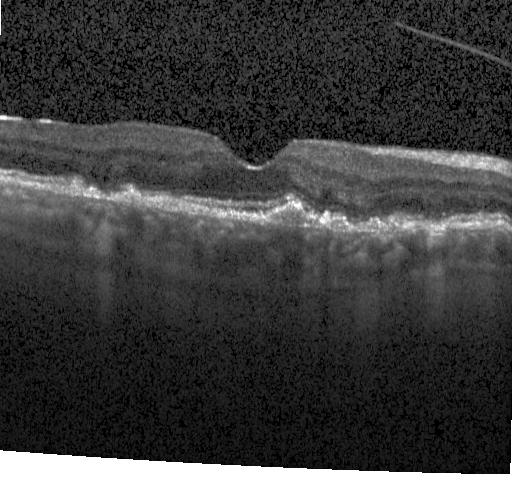

Horizontal scan through the fovea, SD-OCT, acquired on a Heidelberg Spectralis, optical coherence tomography scan. This B-scan demonstrates sub-RPE drusenoid deposits.